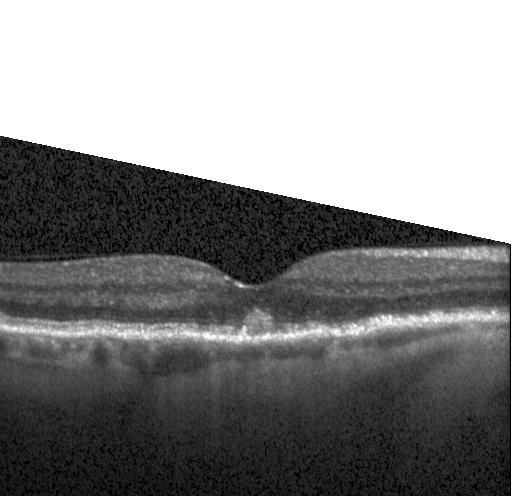

Impression: sub-RPE drusenoid deposits.